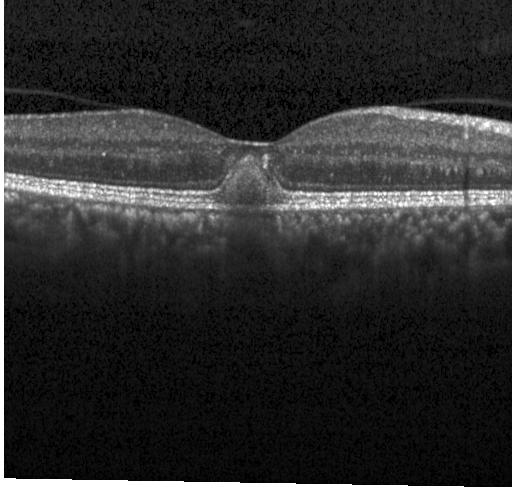 Optical coherence tomography B-scan. Spectral-domain optical coherence tomography — Finding: a choroidal neovascular membrane.